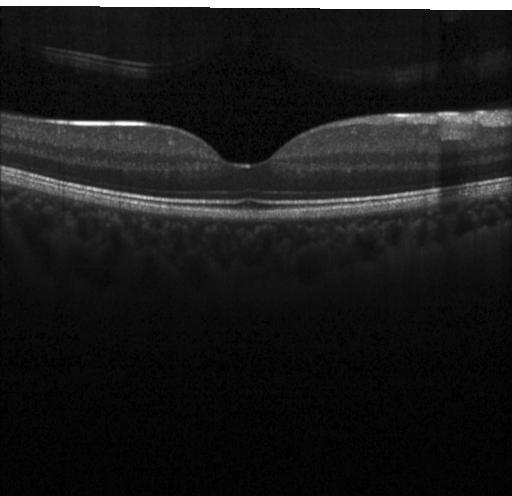

Retinal OCT cross-section; spectral-domain optical coherence tomography
Finding: no choroidal neovascularization, no diabetic macular edema, and no drusen.